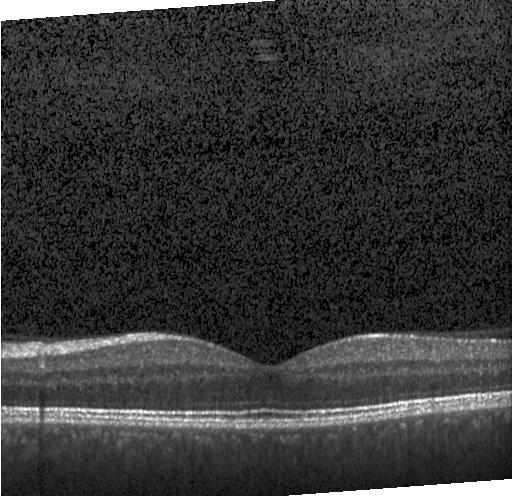 Finding: no choroidal neovascularization, no diabetic macular edema, and no drusen.